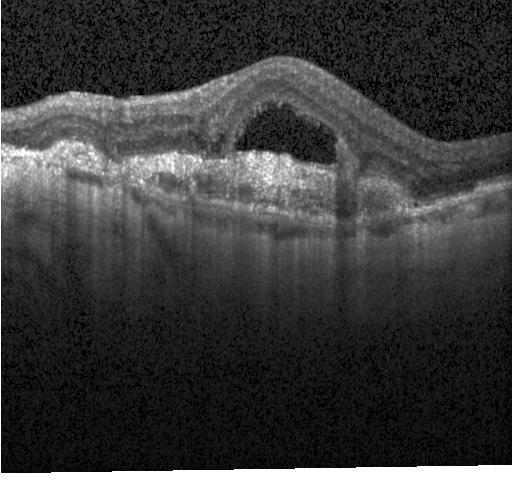
Heidelberg Spectralis, through the macula, retinal OCT B-scan, spectral-domain OCT.
This B-scan demonstrates choroidal neovascularization.